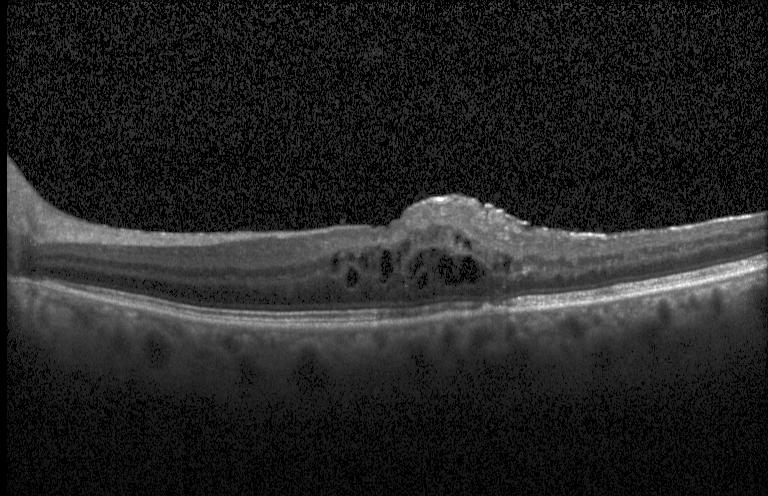

Acquired on a Heidelberg Spectralis; spectral-domain optical coherence tomography; retinal OCT B-scan. The scan shows diabetic macular edema (DME).